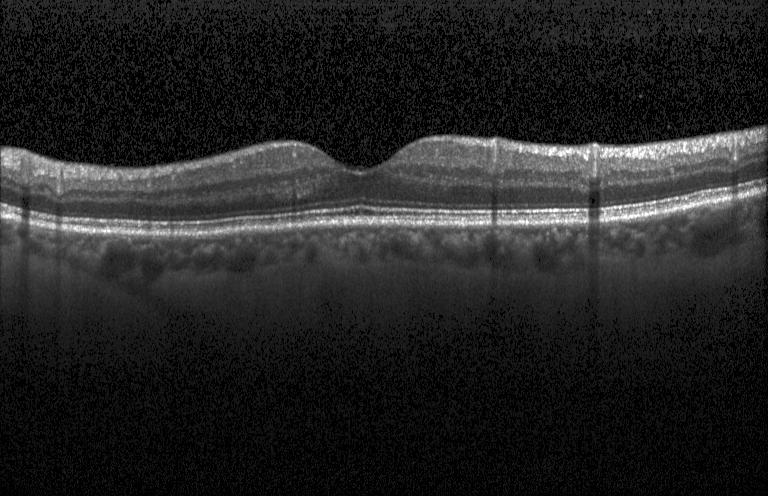

Impression: no choroidal neovascularization, no diabetic macular edema, and no drusen.